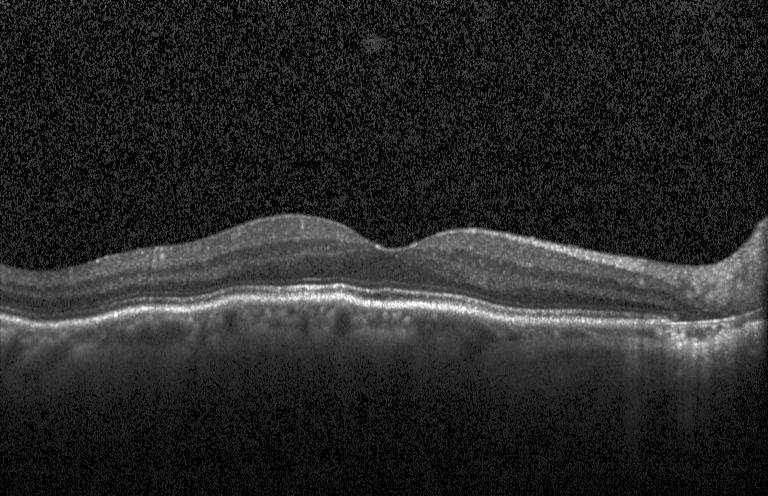
This B-scan demonstrates no choroidal neovascularization, no diabetic macular edema, and no drusen.